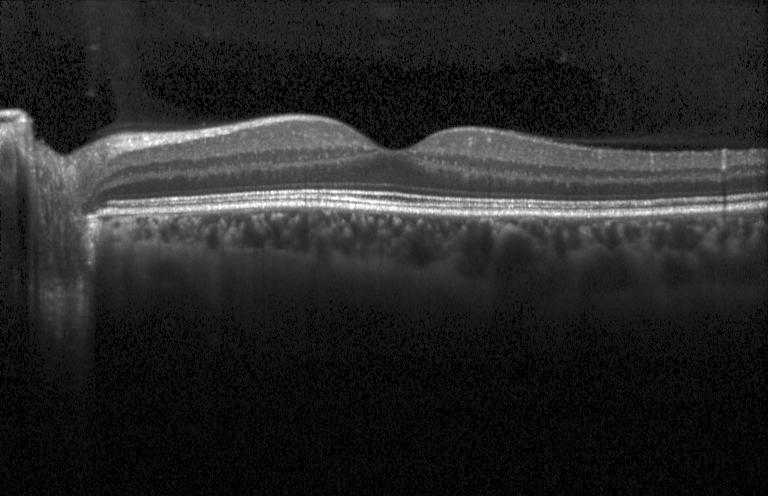 OCT finding: no choroidal neovascularization, no diabetic macular edema, and no drusen.